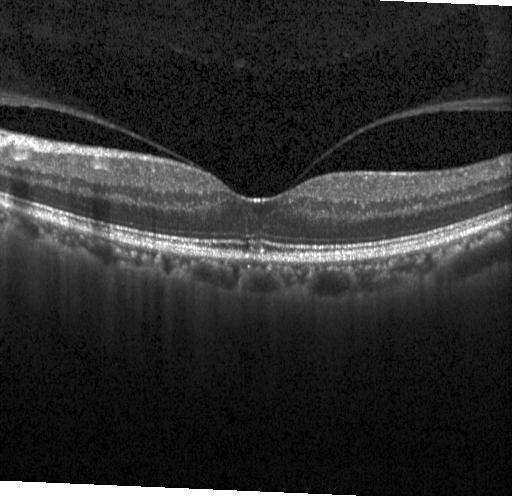
Diabetic macular edema (DME).